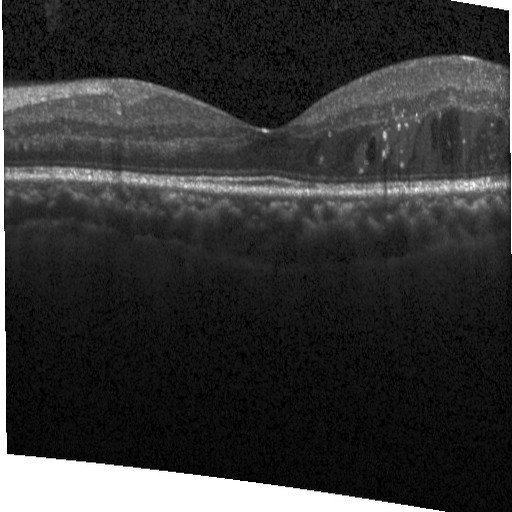 OCT B-scan. This B-scan demonstrates DME.